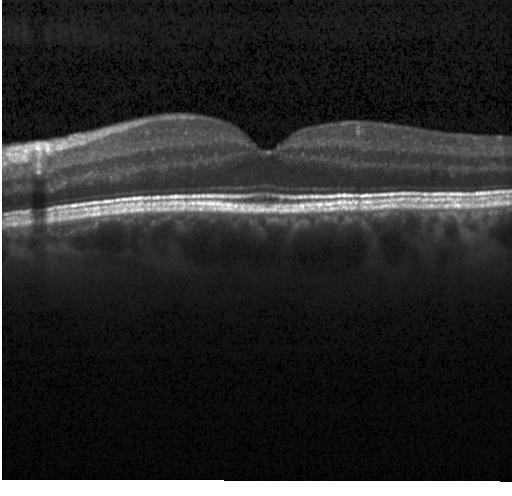 Instrument: Heidelberg Spectralis · retinal OCT cross-section · horizontal scan through the fovea — No CNV, DME, or drusen.